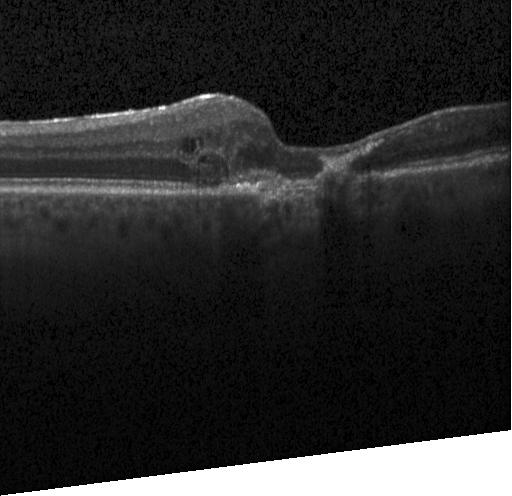 Finding: CNV.